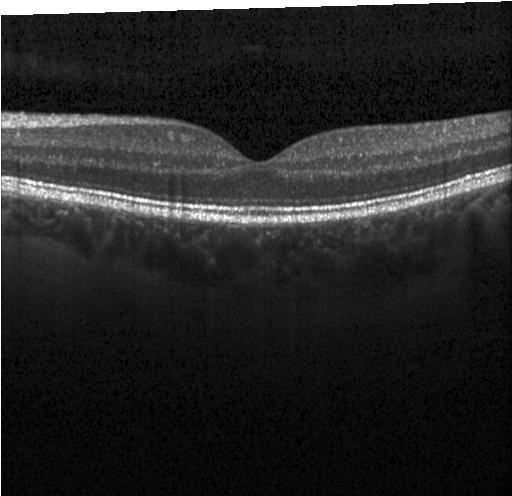
Optical coherence tomography scan · macular scan. Diagnosis: no choroidal neovascularization, diabetic macular edema, or drusen.